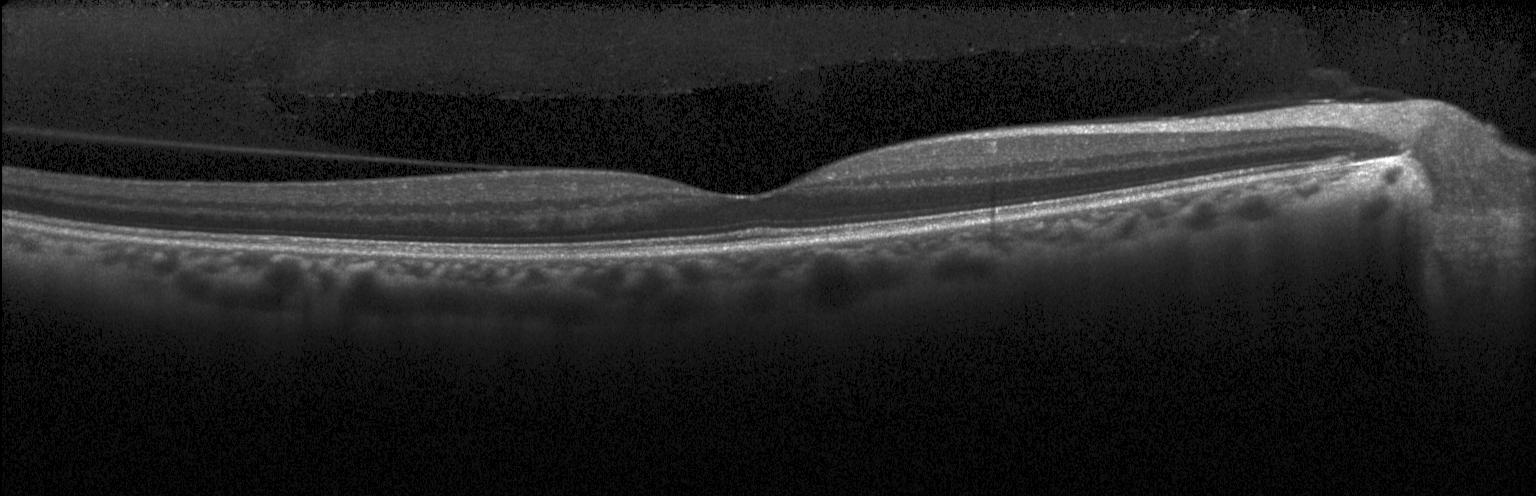 Spectral-domain OCT B-scan: no CNV, no DME, and no drusen.